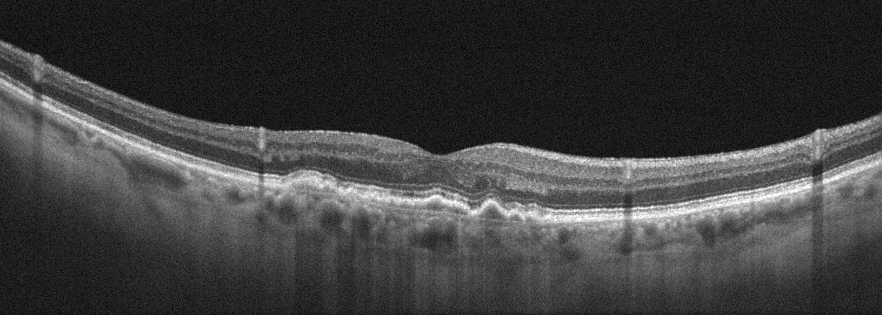
Optical coherence tomography scan; oculus dexter. This B-scan demonstrates age-related macular degeneration.